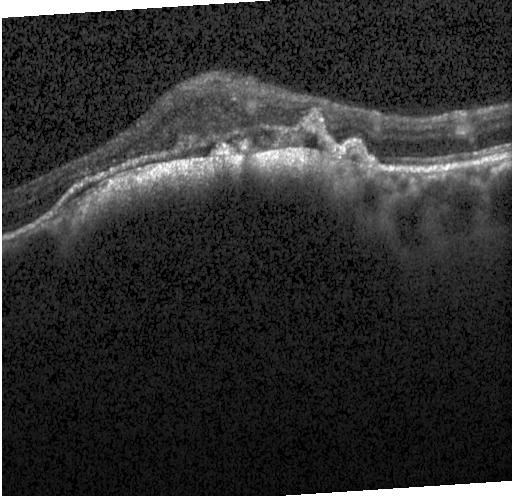 Impression: choroidal neovascularization.